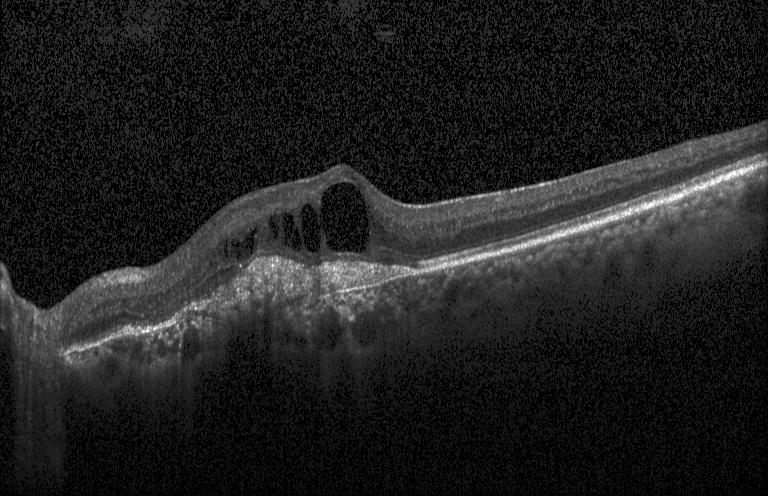
Optical coherence tomography B-scan.
Finding: choroidal neovascularization (CNV).